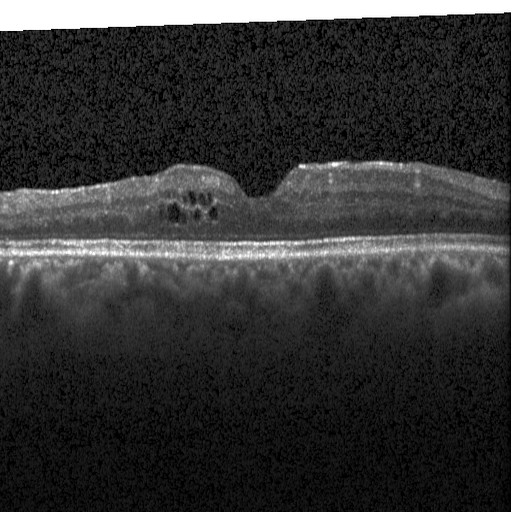

Retinal OCT B-scan · horizontal scan through the fovea — The scan shows diabetic macular edema (DME).